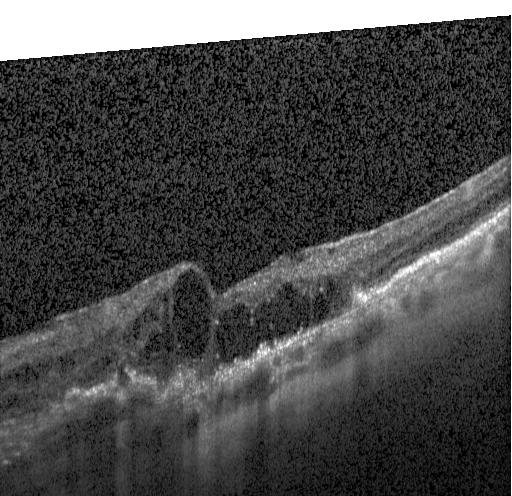

Dx: choroidal neovascularization.